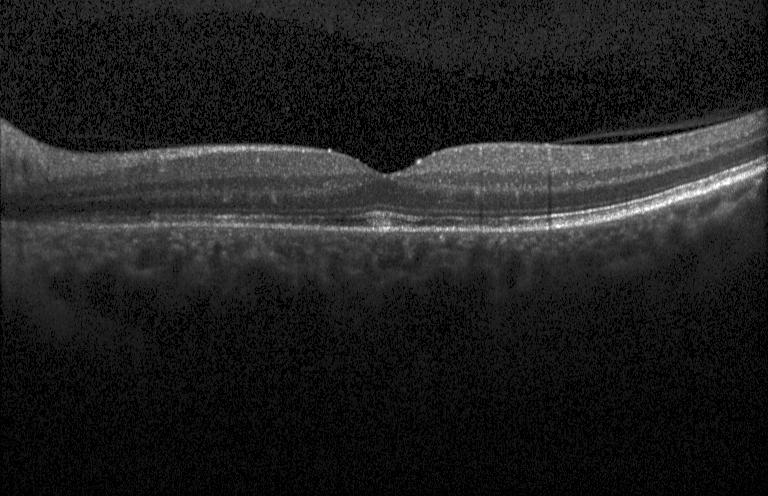 Through the macula. Heidelberg Spectralis OCT system. Retinal OCT B-scan
The scan shows no choroidal neovascularization, diabetic macular edema, or drusen.